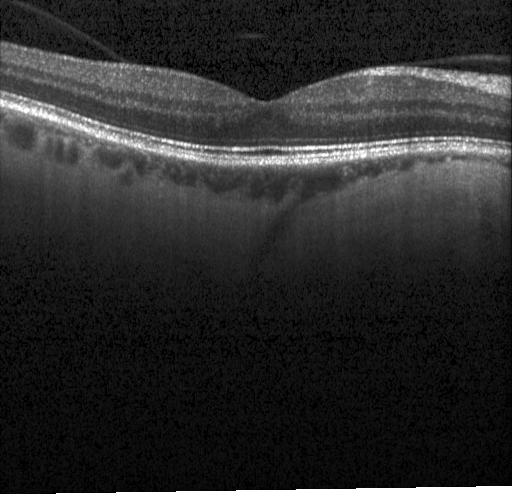
OCT B-scan. Impression: neither CNV, DME, nor drusen.